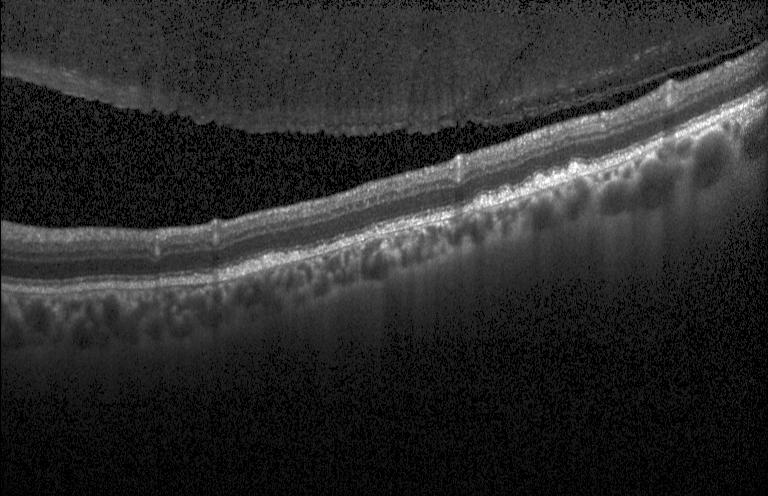

Heidelberg Spectralis OCT system; retinal OCT cross-section
Impression: drusen.